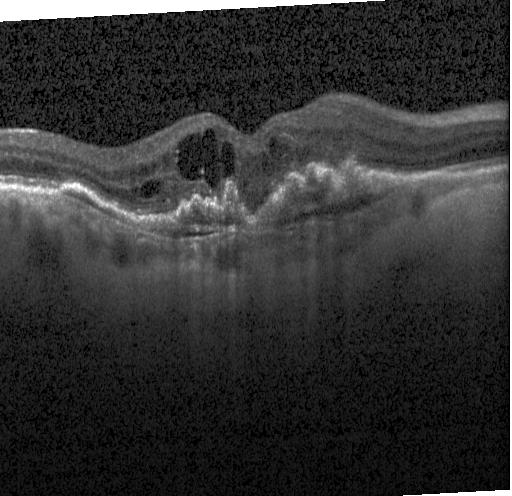

Acquired on a Heidelberg Spectralis. Centered on the fovea. Optical coherence tomography B-scan. Spectral-domain OCT — Finding: CNV.